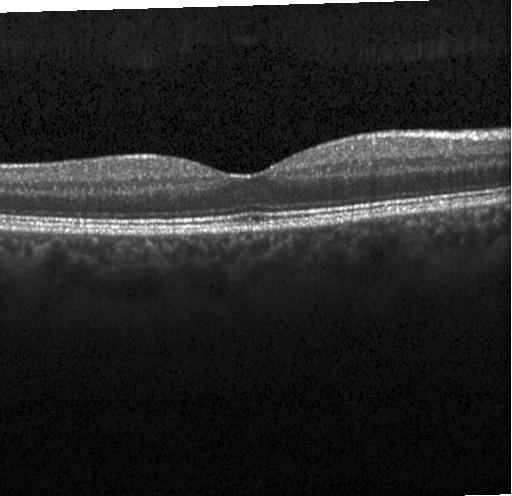 Dx: no evidence of choroidal neovascularization, diabetic macular edema, or drusen.